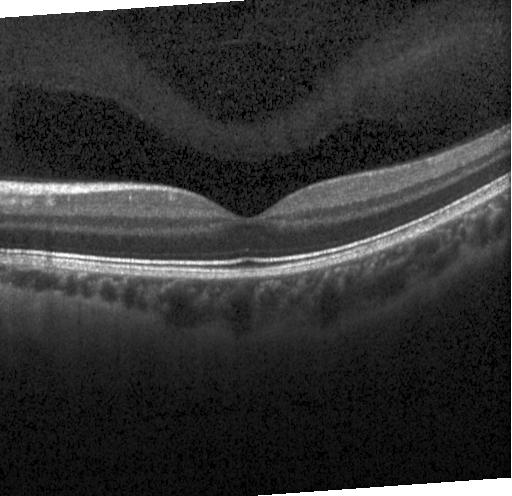 Heidelberg Spectralis OCT system; fovea-centered; retinal OCT cross-section; SD-OCT — This B-scan demonstrates neither choroidal neovascularization, diabetic macular edema, nor drusen.